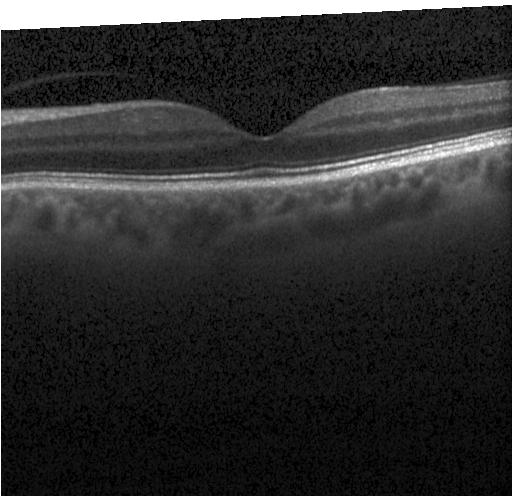 Spectral-domain OCT B-scan: no evidence of CNV, DME, or drusen.